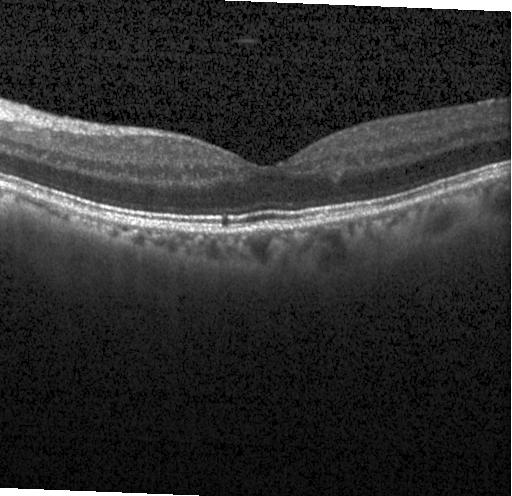
SD-OCT. Through the macula. Acquired on a Heidelberg Spectralis. OCT B-scan
Neither choroidal neovascularization, diabetic macular edema, nor drusen.